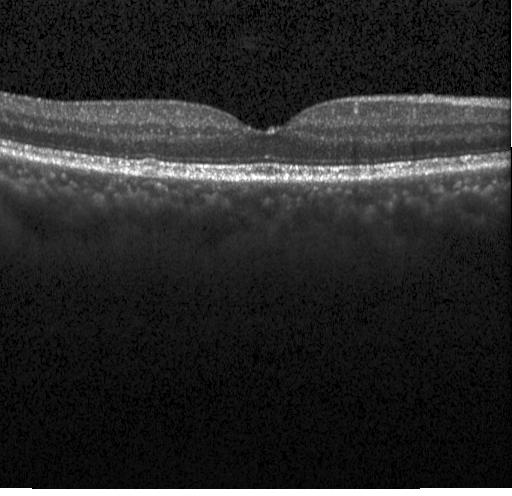 Spectral-domain OCT; OCT B-scan
The scan shows multiple drusen.